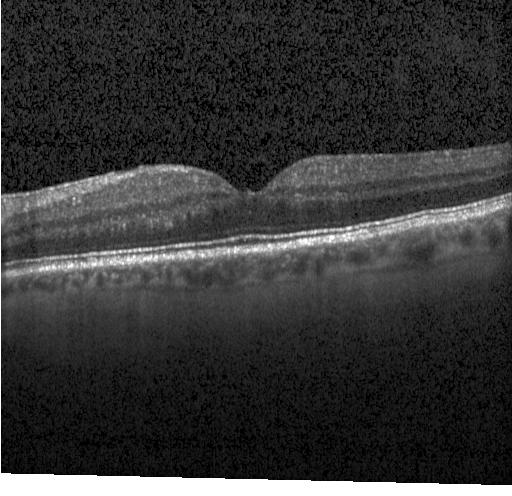
Fovea-centered. SD-OCT. Acquired on a Heidelberg Spectralis. OCT B-scan.
No choroidal neovascularization, diabetic macular edema, or drusen.